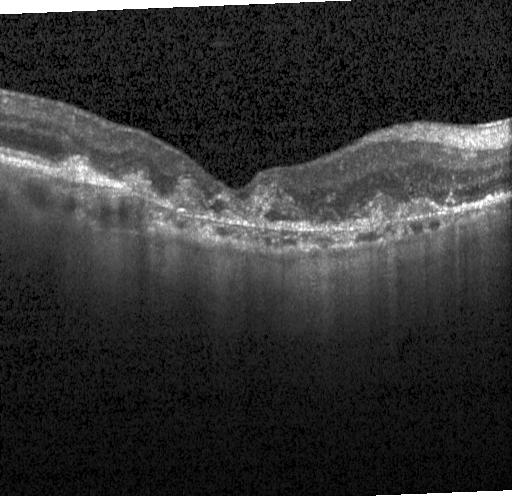 Dx: a choroidal neovascular membrane.